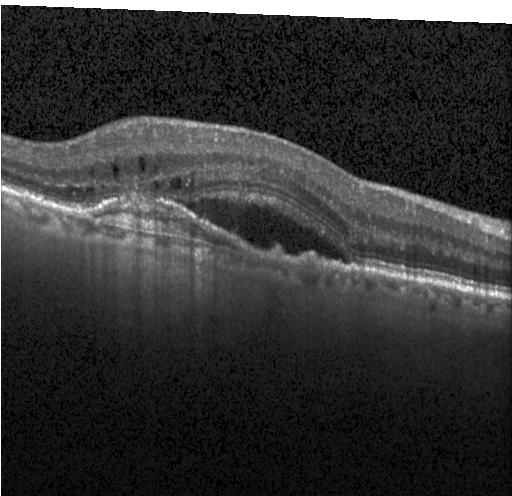 Impression: a choroidal neovascular membrane.